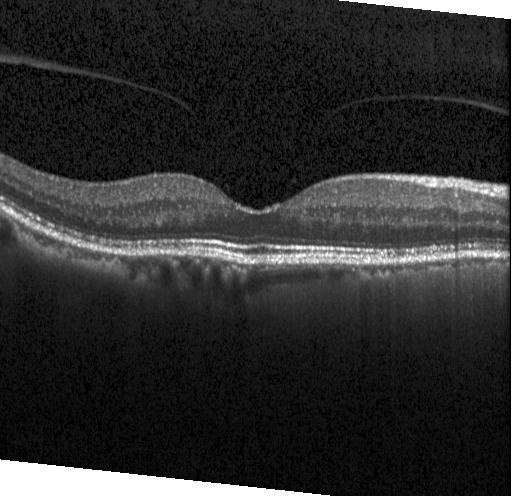
Optical coherence tomography scan · fovea-centered · Heidelberg Spectralis OCT system · spectral-domain OCT. Diagnosis: neither choroidal neovascularization, diabetic macular edema, nor drusen.